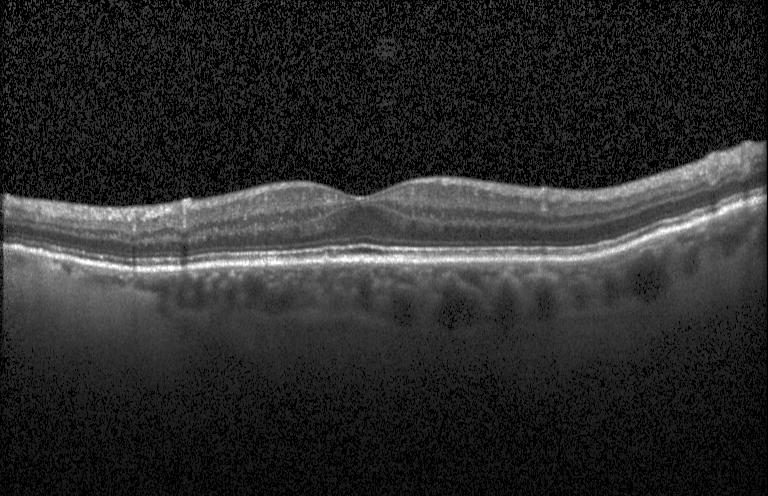
Optical coherence tomography B-scan.
Impression: no CNV, DME, or drusen.